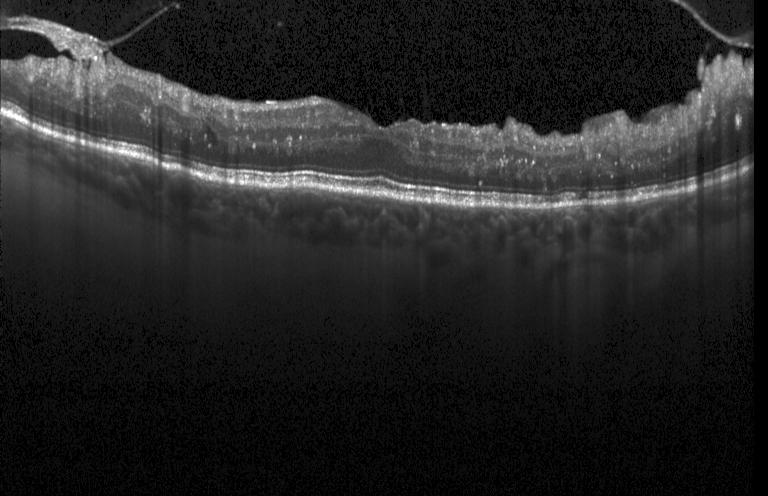
Optical coherence tomography scan. Impression: DME.